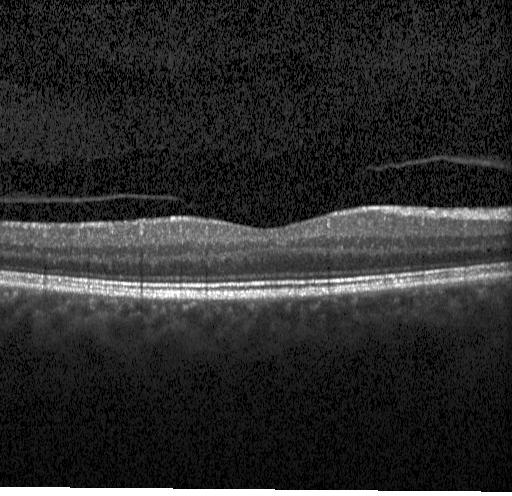

OCT B-scan.
Dx: no choroidal neovascularization, diabetic macular edema, or drusen.